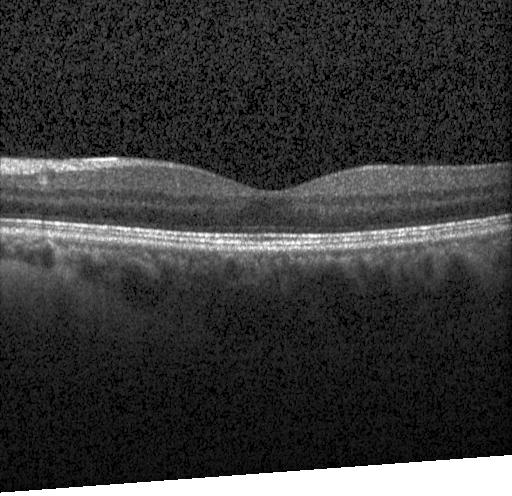

Spectral-domain OCT; retinal OCT B-scan; acquired on a Heidelberg Spectralis; horizontal scan through the fovea.
Impression: no CNV, DME, or drusen.